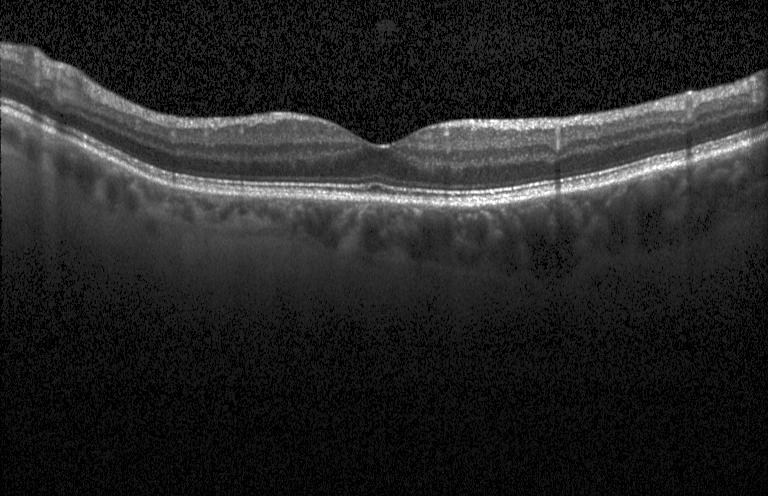
Finding: no evidence of CNV, DME, or drusen.